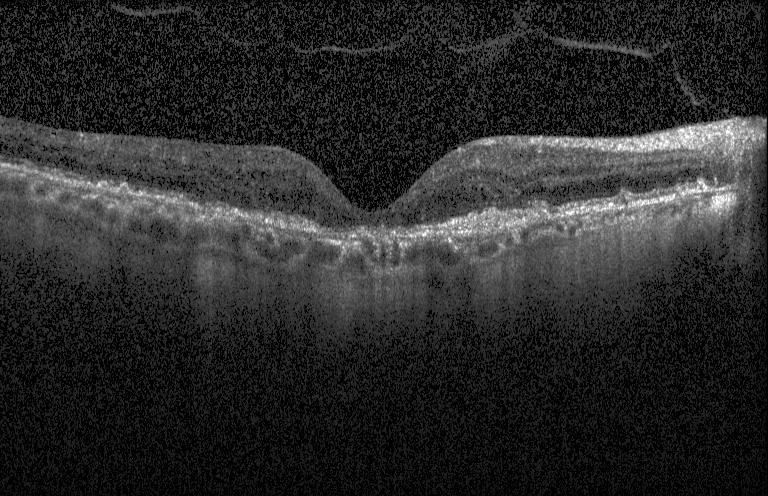

Optical coherence tomography B-scan
Diagnosis: a choroidal neovascular membrane.